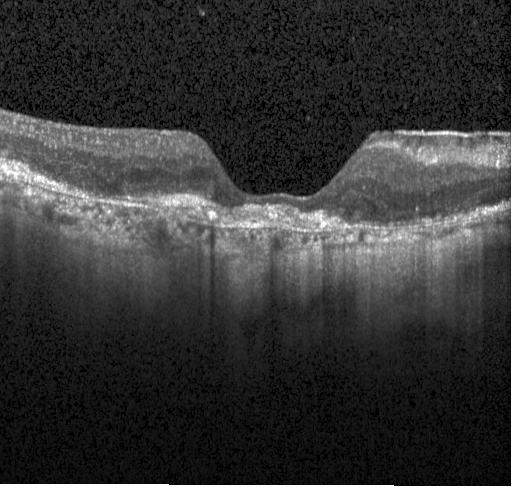 Macular OCT: a choroidal neovascular membrane.